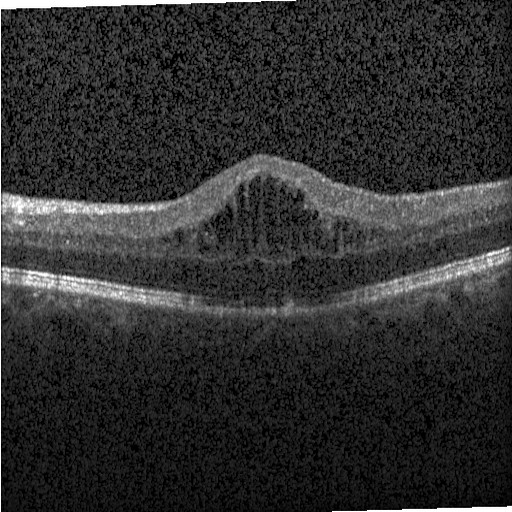 OCT B-scan.
Diagnosis: diabetic macular edema.